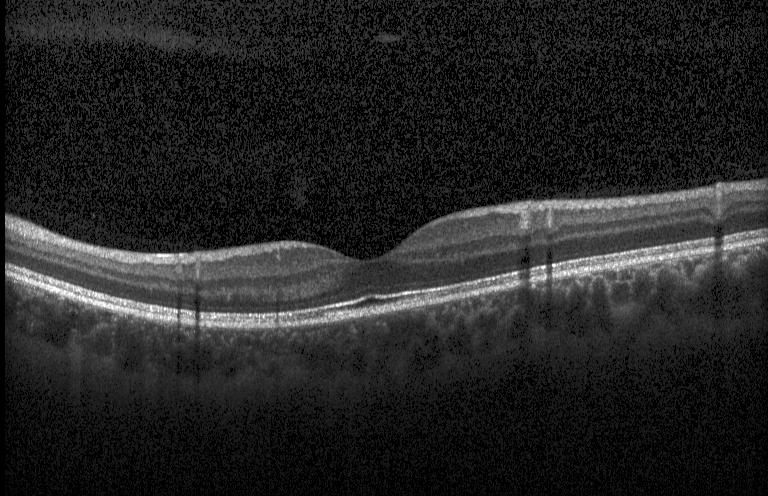

Retinal OCT cross-section — Impression: no choroidal neovascularization, diabetic macular edema, or drusen.